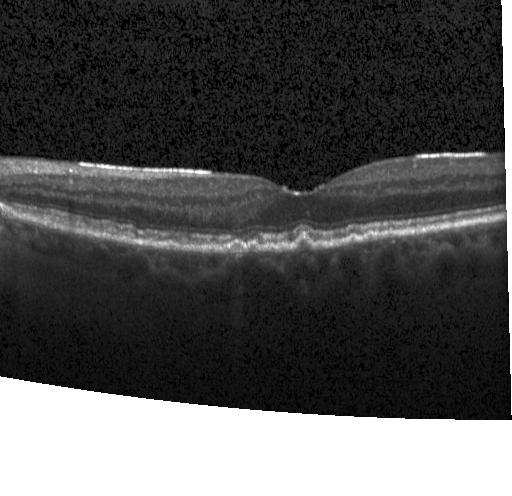

Spectral-domain OCT. Acquired on a Heidelberg Spectralis. Macular scan. Optical coherence tomography B-scan — Drusen.